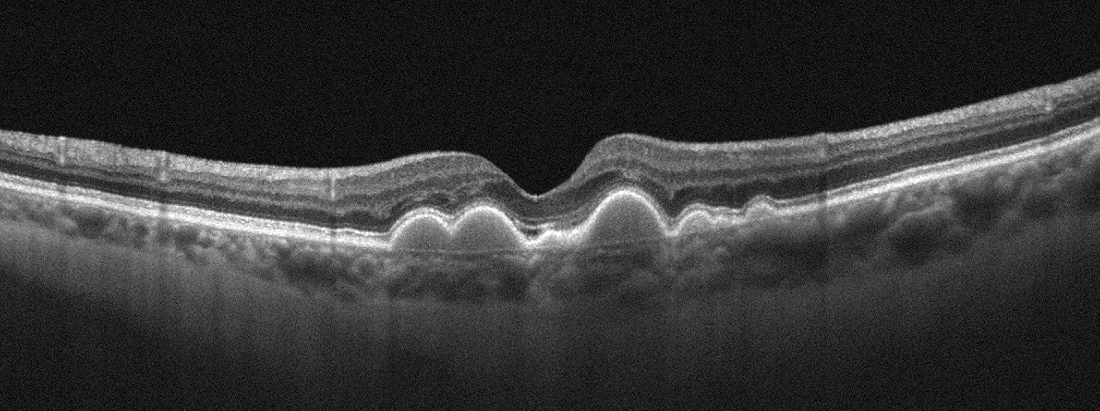 Spectral-domain OCT B-scan: age-related macular degeneration.